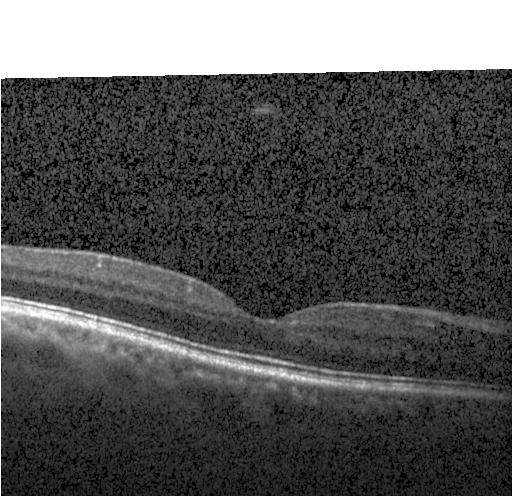
Optical coherence tomography scan. Impression: no choroidal neovascularization, diabetic macular edema, or drusen.